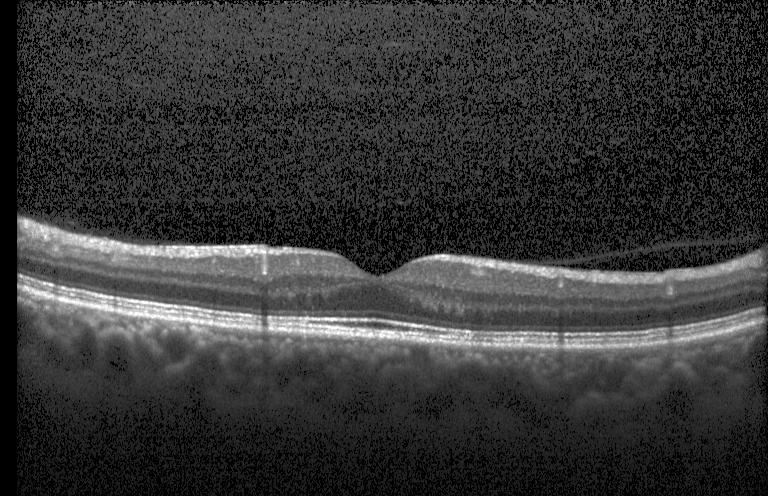 Optical coherence tomography B-scan.
OCT finding: no evidence of CNV, DME, or drusen.